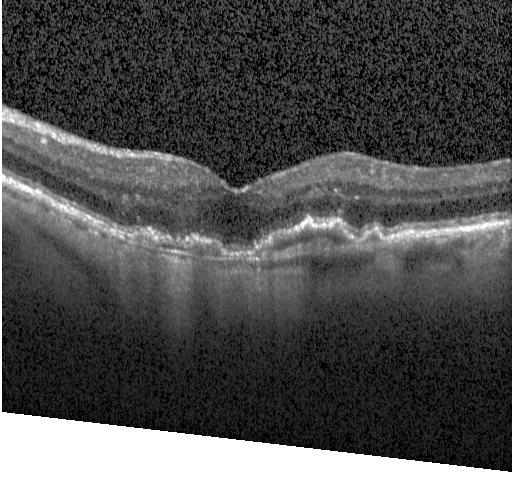 Retinal OCT cross-section. Finding: CNV.